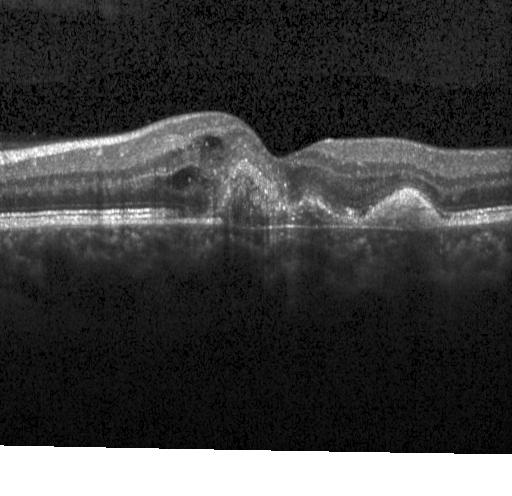 Macular OCT demonstrating choroidal neovascularization.